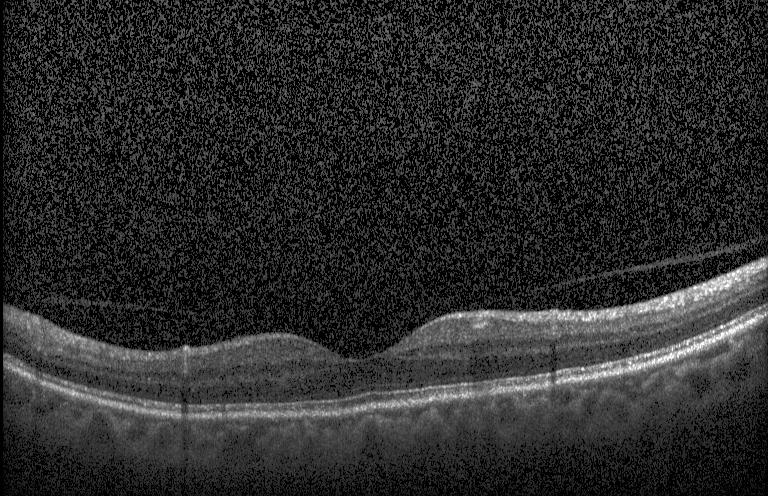
Through the macula, retinal OCT B-scan. Finding: no evidence of choroidal neovascularization, diabetic macular edema, or drusen.